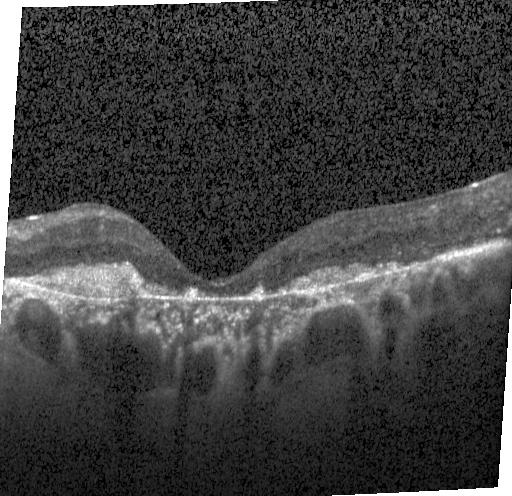 Macular OCT demonstrating a choroidal neovascular membrane.